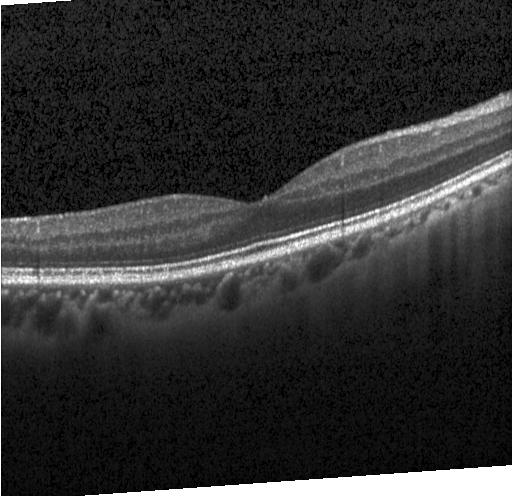
OCT B-scan — No CNV, DME, or drusen.